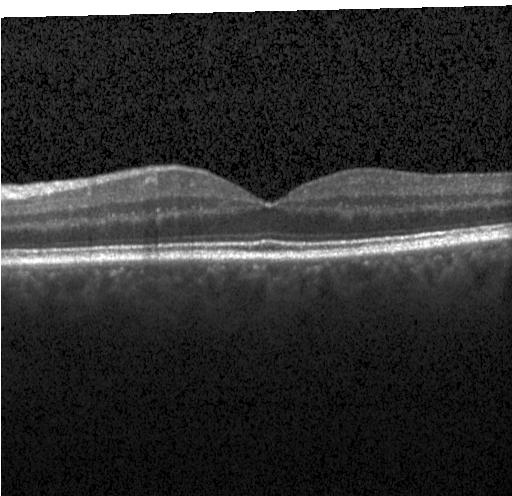
Finding: no choroidal neovascularization, no diabetic macular edema, and no drusen.